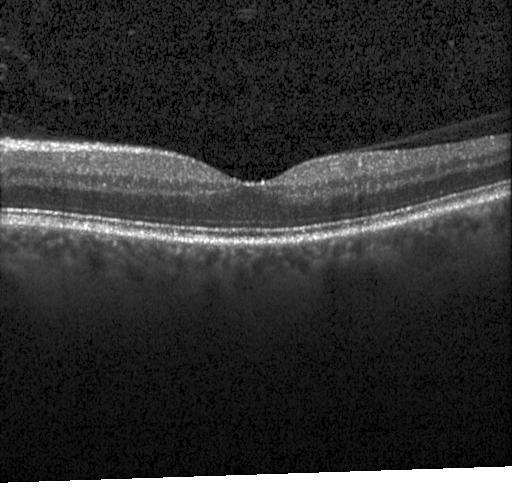 Impression: no CNV, no DME, and no drusen.